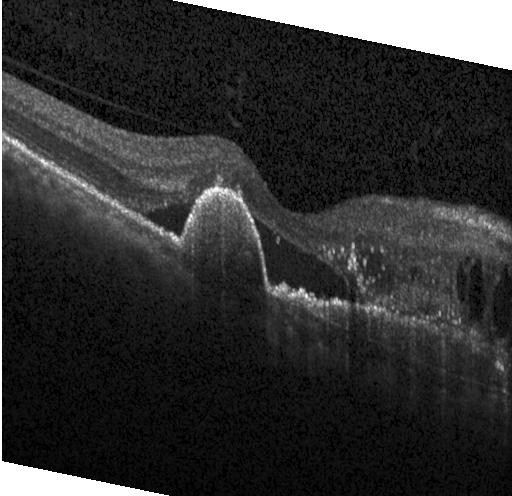
Retinal OCT B-scan — Diagnosis: a choroidal neovascular membrane.